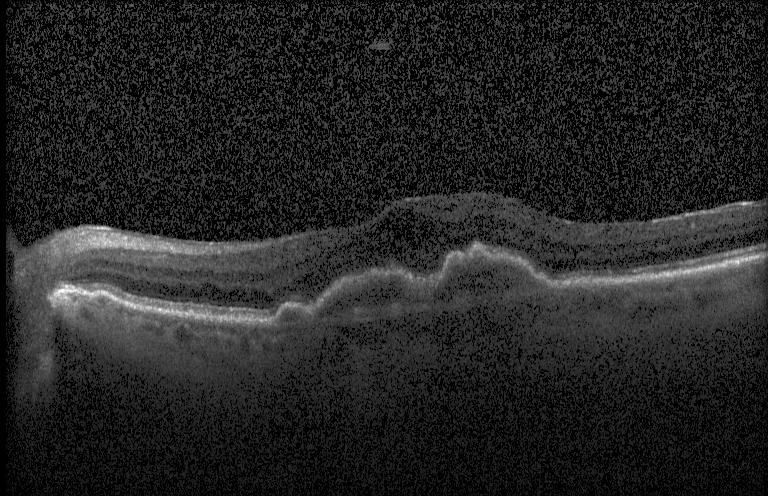 Retinal OCT B-scan, spectral-domain optical coherence tomography
Finding: a choroidal neovascular membrane.